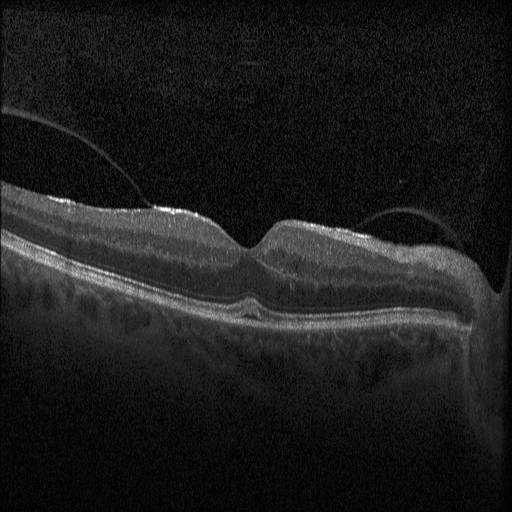

OCT line scan — Finding: diabetic macular edema.